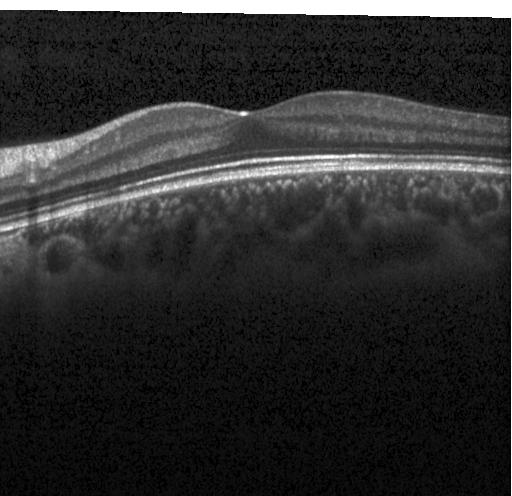

Spectral-domain optical coherence tomography, OCT line scan. Impression: no choroidal neovascularization, no diabetic macular edema, and no drusen.